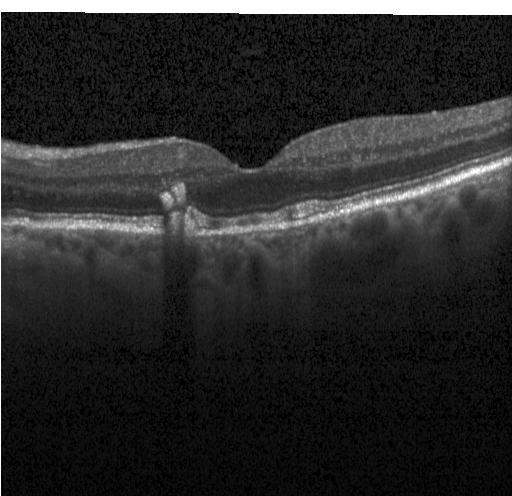
Spectral-domain optical coherence tomography · fovea-centered · retinal OCT B-scan. Assessment: sub-RPE drusenoid deposits.